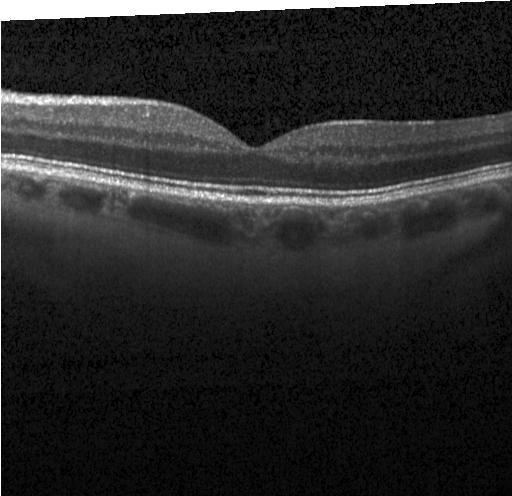

Diagnosis: no CNV, DME, or drusen.